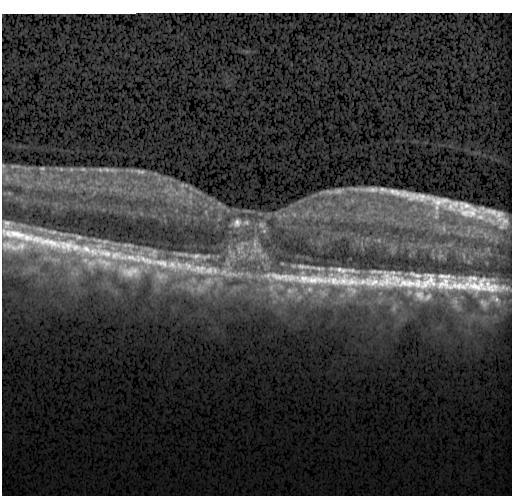

Spectral-domain OCT · optical coherence tomography scan
Assessment: a choroidal neovascular membrane.